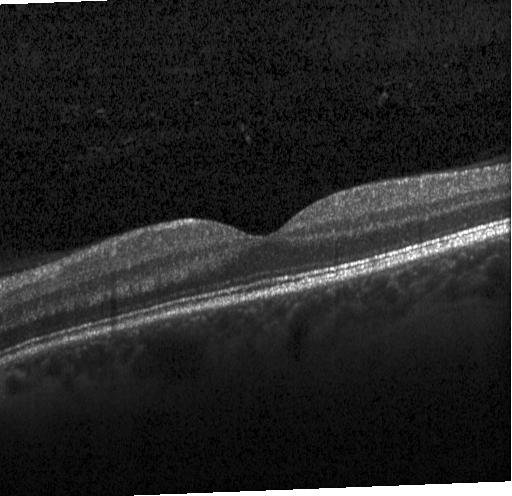 OCT B-scan — Assessment: no CNV, no DME, and no drusen.